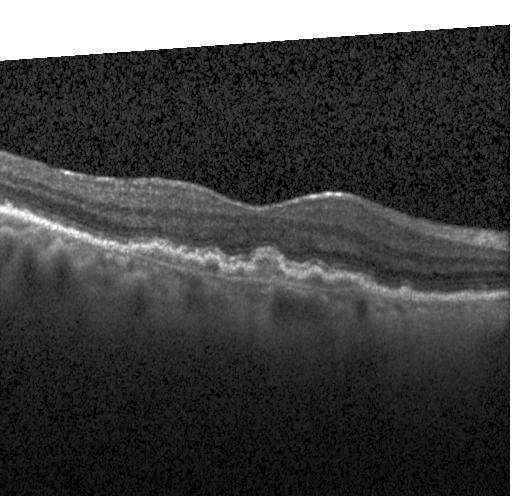

CNV.